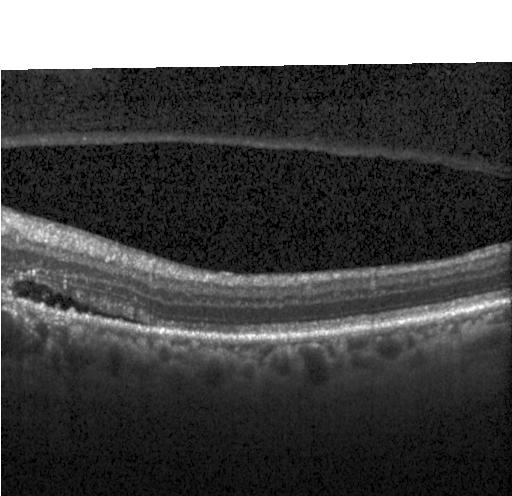 The scan shows choroidal neovascularization.